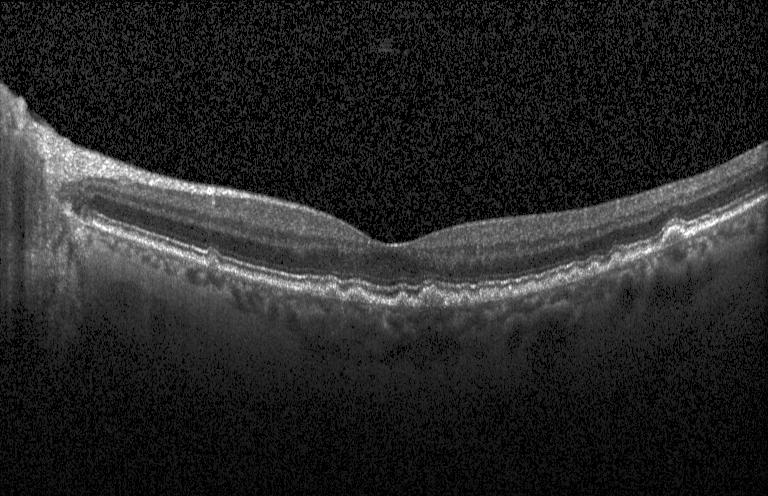
Macular OCT: multiple drusen.